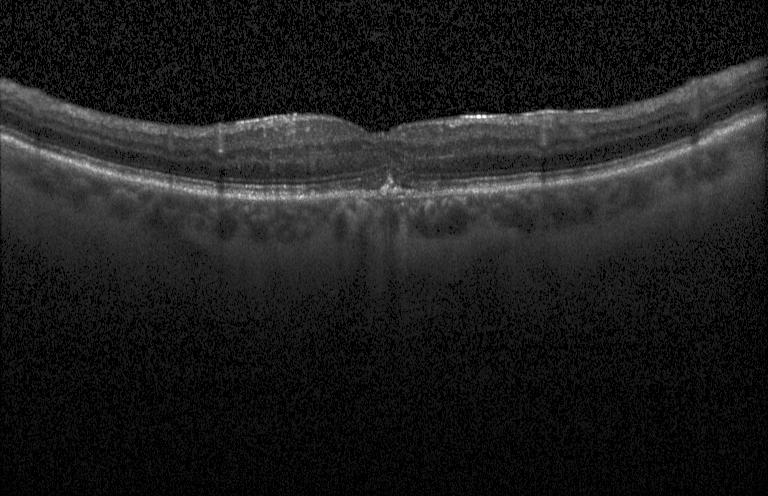
Spectral-domain OCT B-scan: a choroidal neovascular membrane.